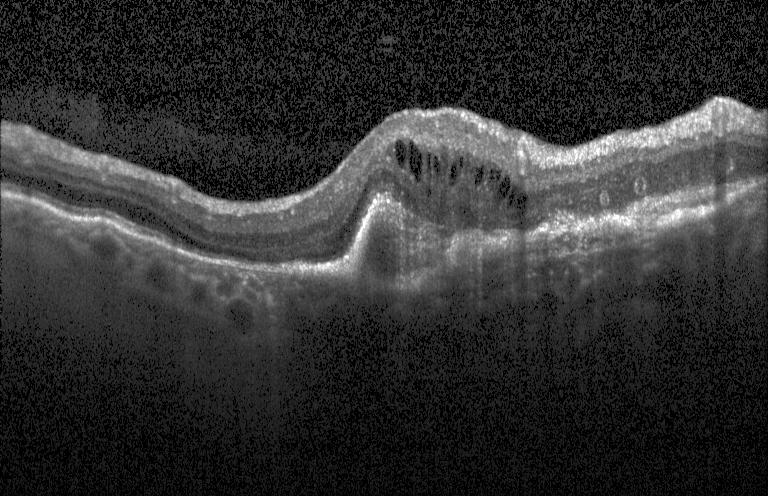

Spectral-domain OCT. Optical coherence tomography B-scan — This B-scan demonstrates a choroidal neovascular membrane.